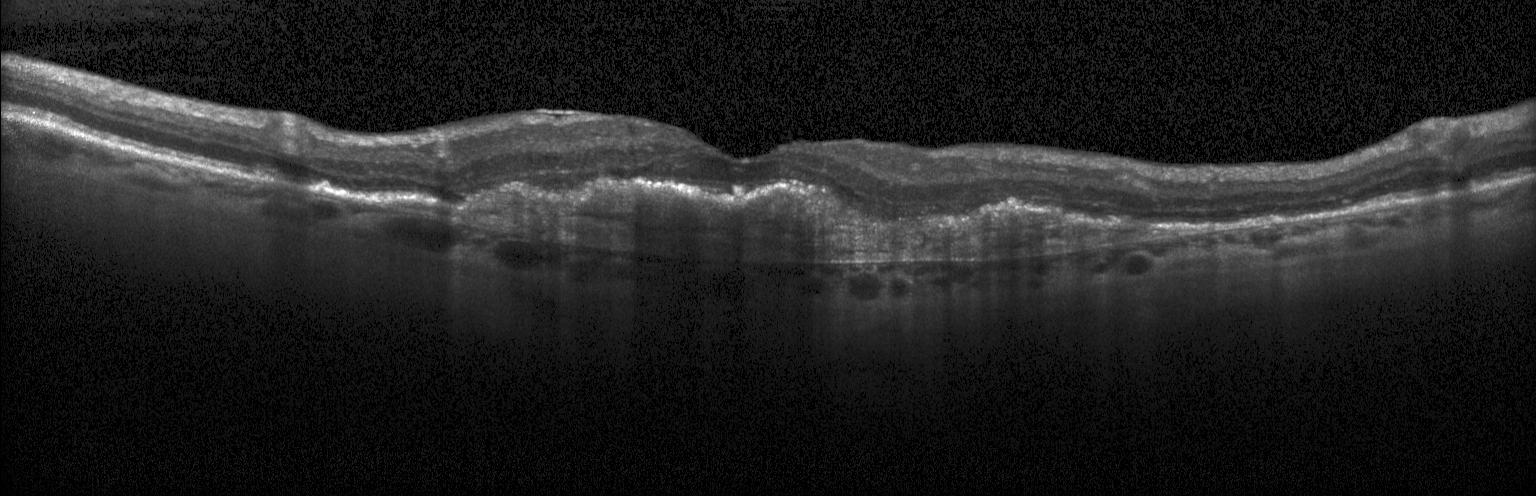
This B-scan demonstrates choroidal neovascularization.